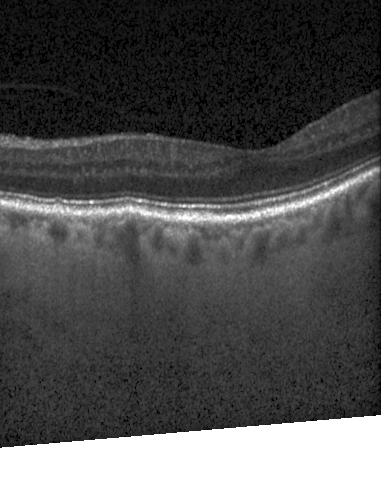

Through the macula. OCT B-scan.
Impression: no CNV, no DME, and no drusen.